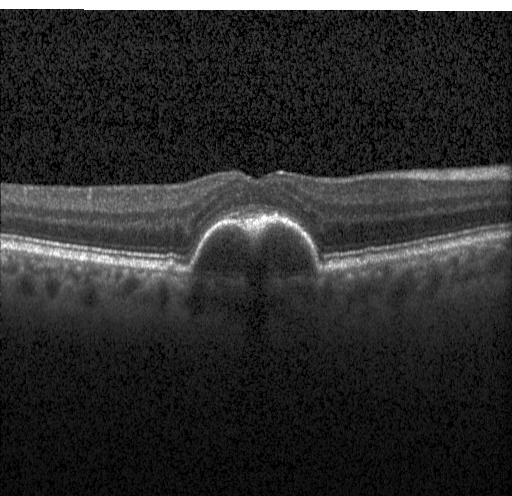
Fovea-centered · optical coherence tomography B-scan — Macular OCT: a choroidal neovascular membrane.